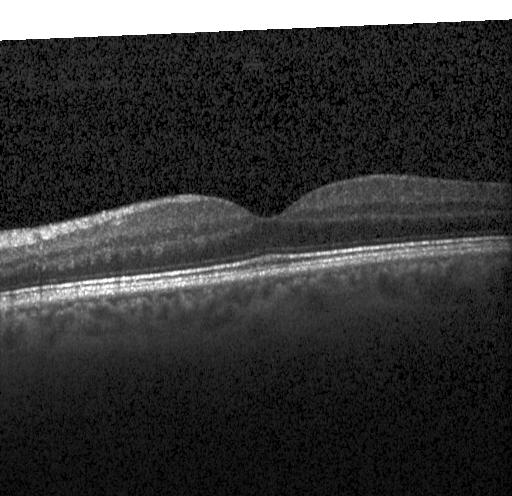 Spectral-domain OCT B-scan: no choroidal neovascularization, diabetic macular edema, or drusen.